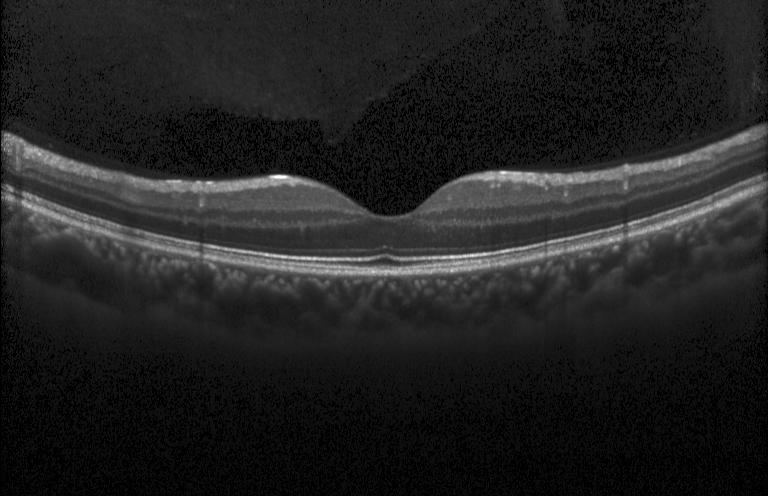 Finding: no choroidal neovascularization, no diabetic macular edema, and no drusen.